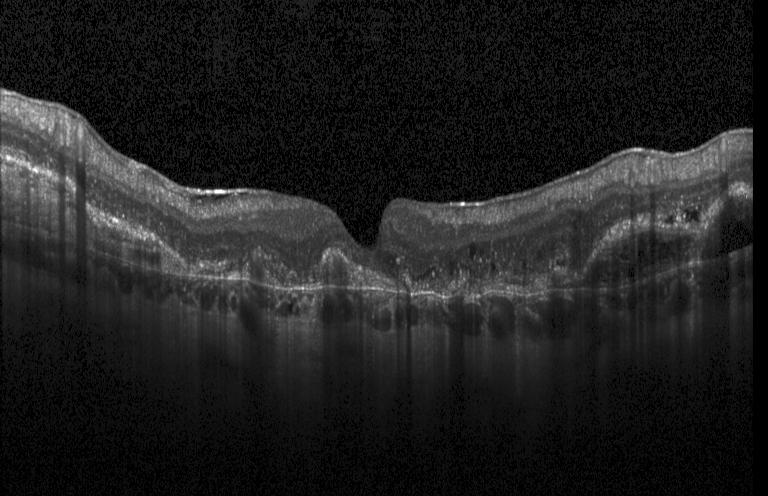

OCT scan showing choroidal neovascularization (CNV).